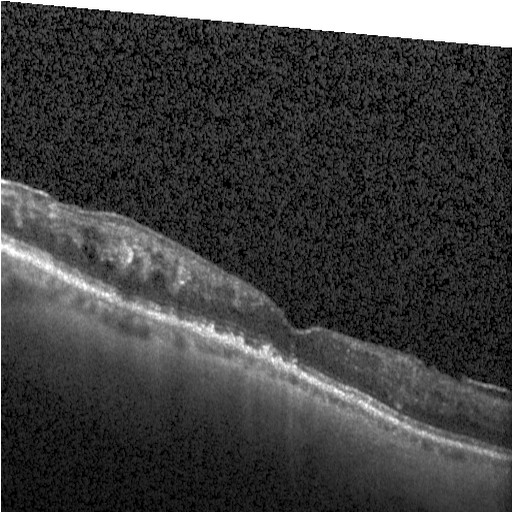
Assessment: DME.